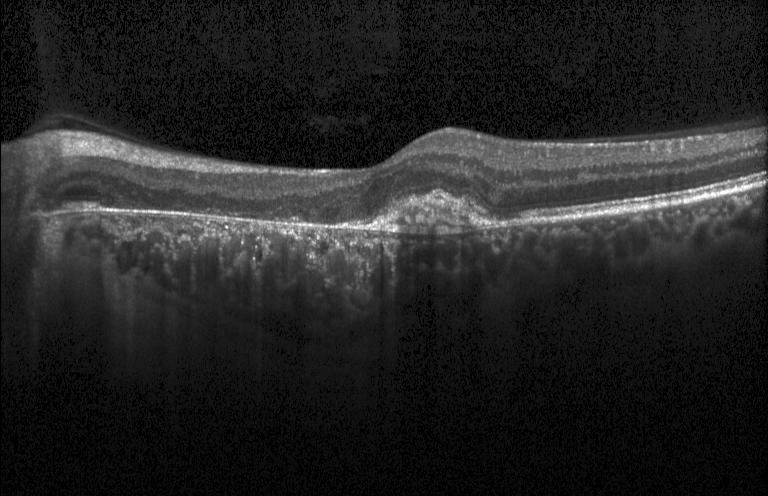 Optical coherence tomography B-scan — Diagnosis: a choroidal neovascular membrane.